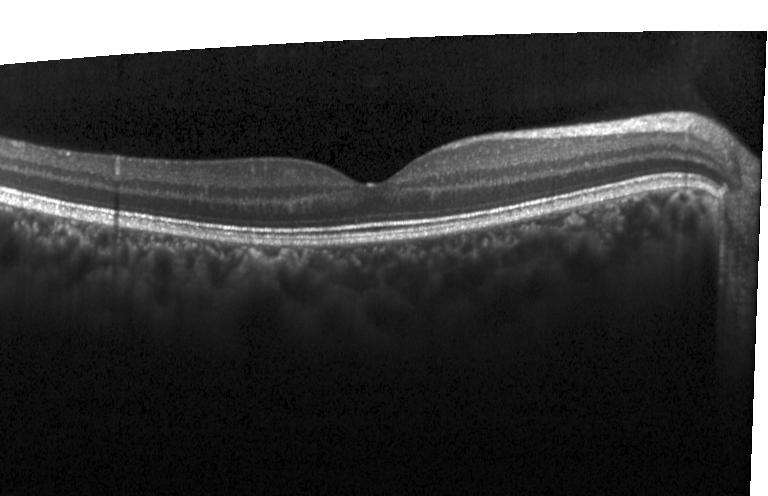
Optical coherence tomography scan; horizontal scan through the fovea; Heidelberg Spectralis OCT system. OCT finding: no CNV, DME, or drusen.